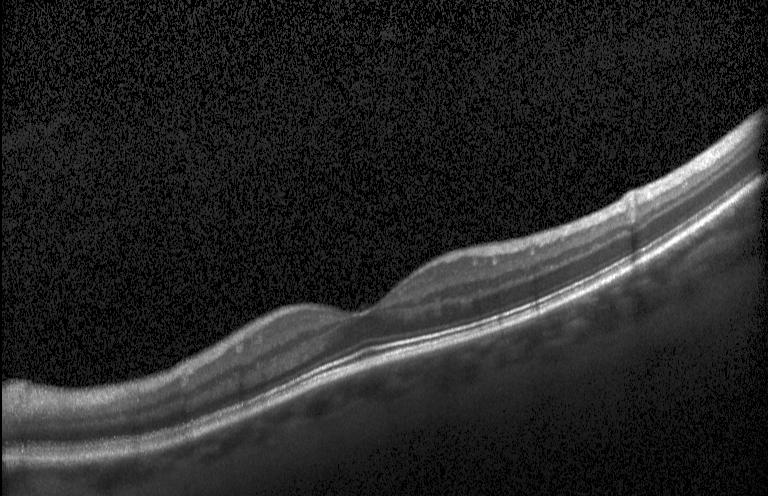
Optical coherence tomography B-scan, spectral-domain optical coherence tomography — Dx: no choroidal neovascularization, diabetic macular edema, or drusen.